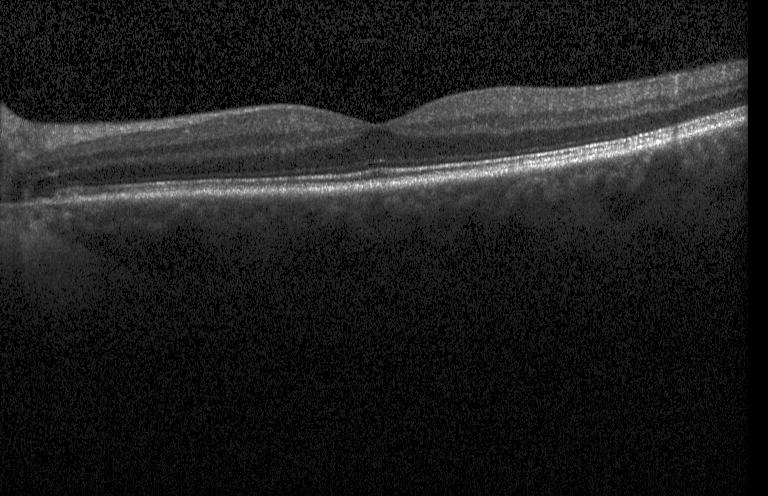

Spectral-domain optical coherence tomography. Fovea-centered. Acquired on a Heidelberg Spectralis. OCT B-scan — Finding: no evidence of CNV, DME, or drusen.